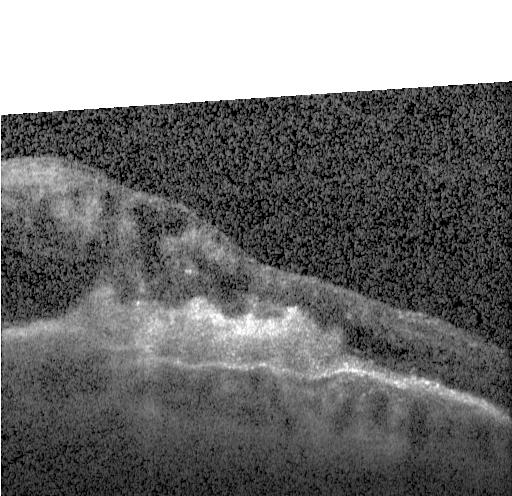

Optical coherence tomography B-scan · Heidelberg Spectralis OCT system · spectral-domain optical coherence tomography · macular scan.
Diagnosis: a choroidal neovascular membrane.